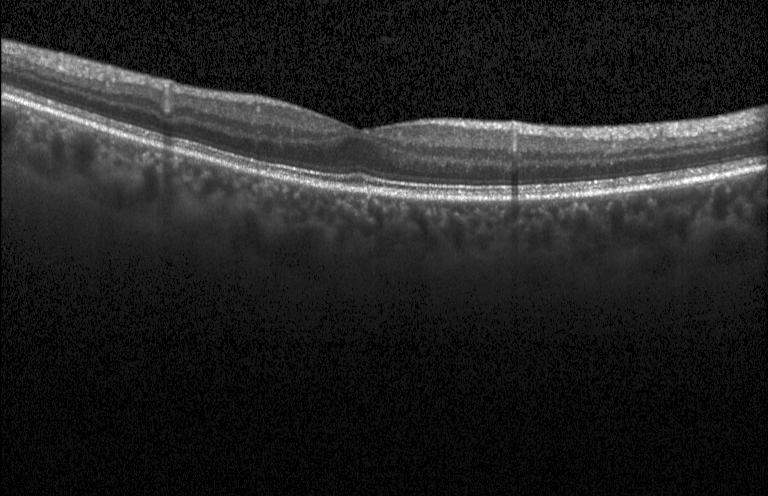

OCT B-scan showing no choroidal neovascularization, no diabetic macular edema, and no drusen.